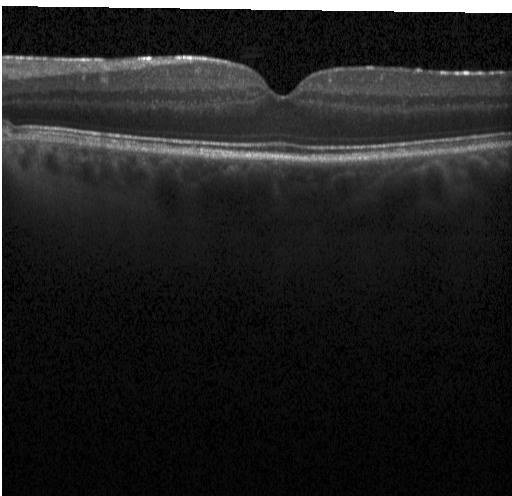

Retinal OCT cross-section. Through the macula
Diagnosis: neither choroidal neovascularization, diabetic macular edema, nor drusen.